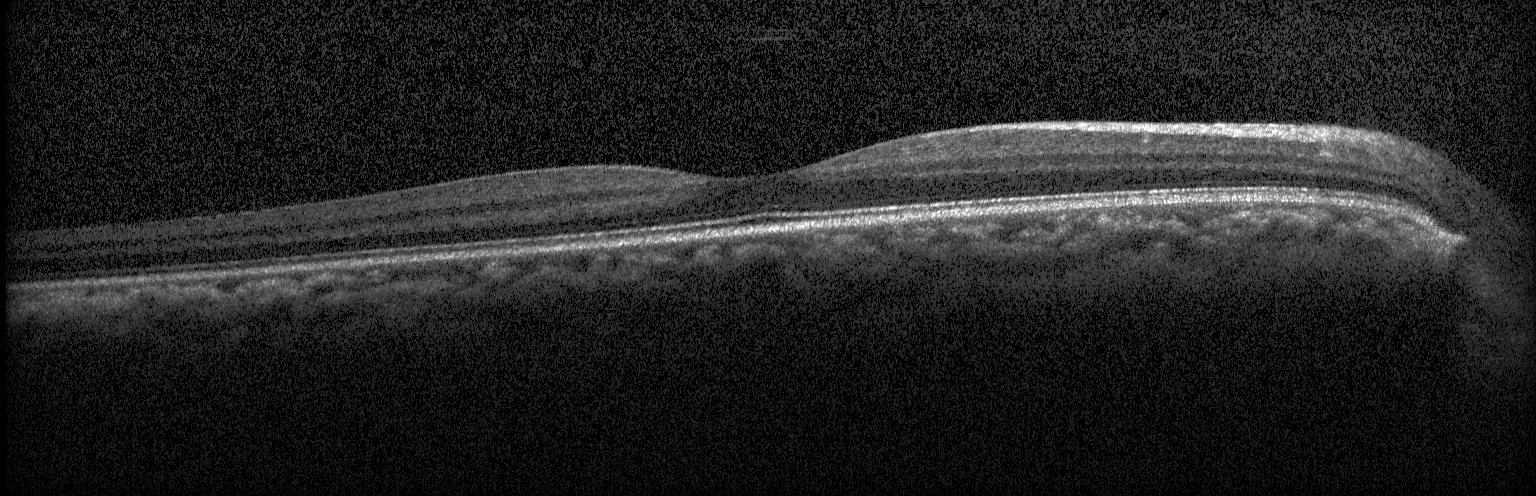
Optical coherence tomography scan. Through the macula. Instrument: Heidelberg Spectralis
Impression: no choroidal neovascularization, no diabetic macular edema, and no drusen.